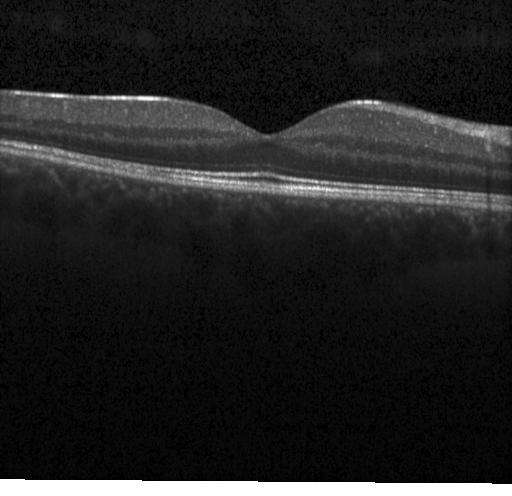

No choroidal neovascularization, diabetic macular edema, or drusen.